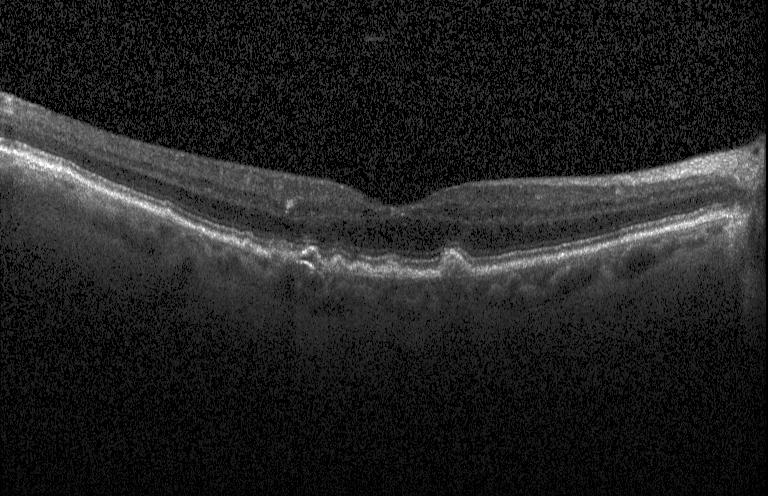
Optical coherence tomography B-scan; spectral-domain optical coherence tomography — This B-scan demonstrates sub-RPE drusenoid deposits.